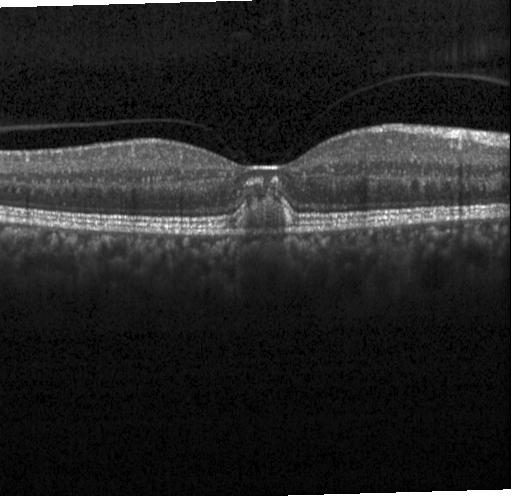

Macular OCT demonstrating a choroidal neovascular membrane.